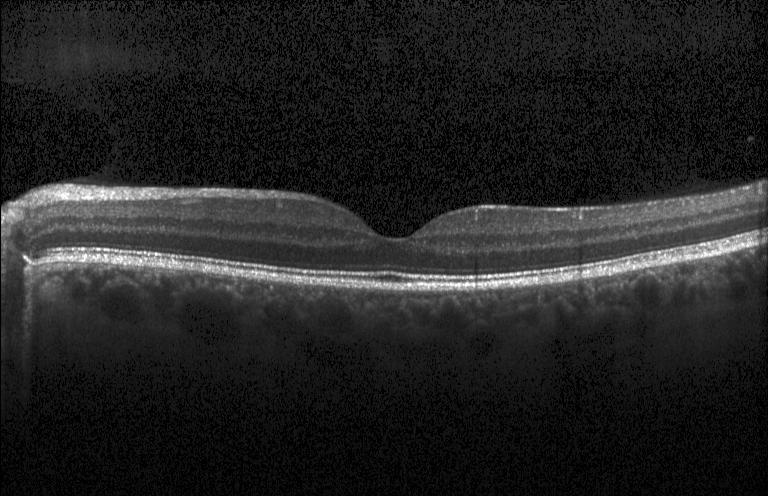 OCT B-scan.
The scan shows neither choroidal neovascularization, diabetic macular edema, nor drusen.